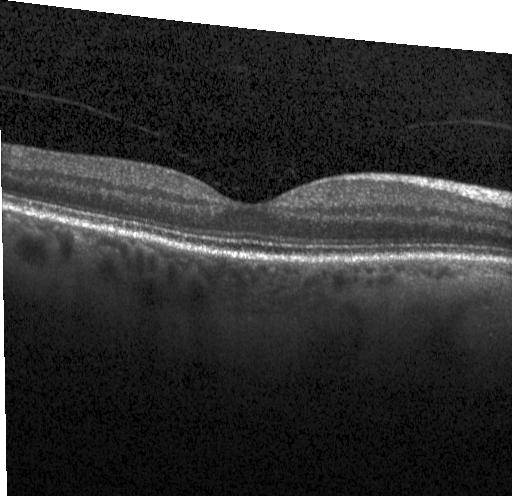
Spectral-domain optical coherence tomography; optical coherence tomography B-scan. No choroidal neovascularization, no diabetic macular edema, and no drusen.